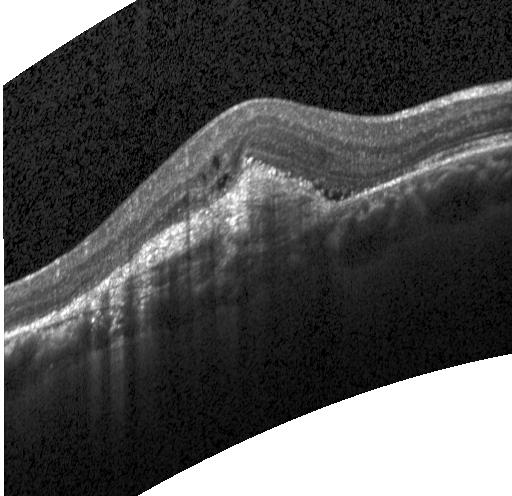
Dx: CNV.